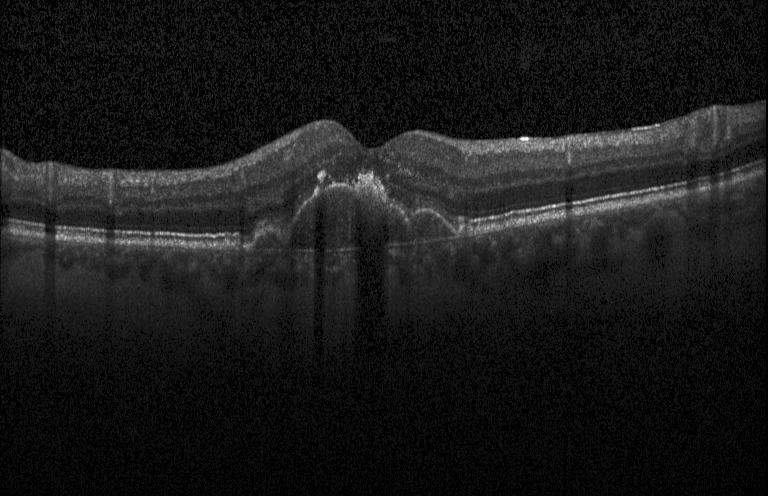
Fovea-centered; Heidelberg Spectralis OCT system; optical coherence tomography scan.
Diagnosis: a choroidal neovascular membrane.